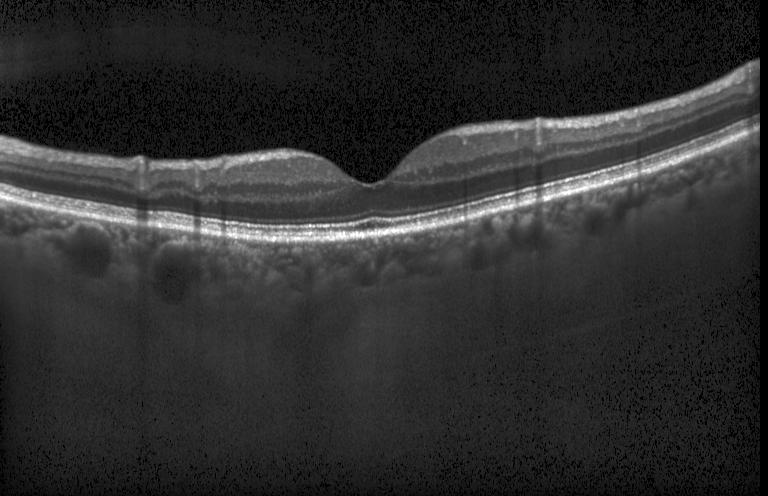
Spectral-domain OCT. Centered on the fovea. Instrument: Heidelberg Spectralis. Optical coherence tomography B-scan. No CNV, no DME, and no drusen.